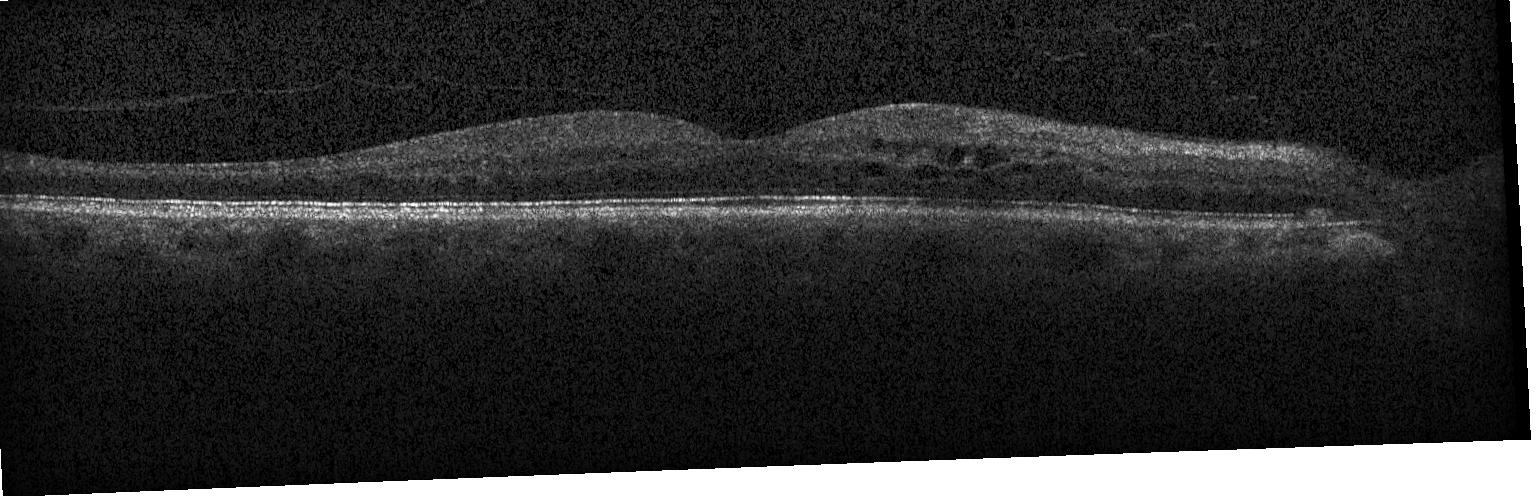 OCT finding: diabetic macular edema (DME).